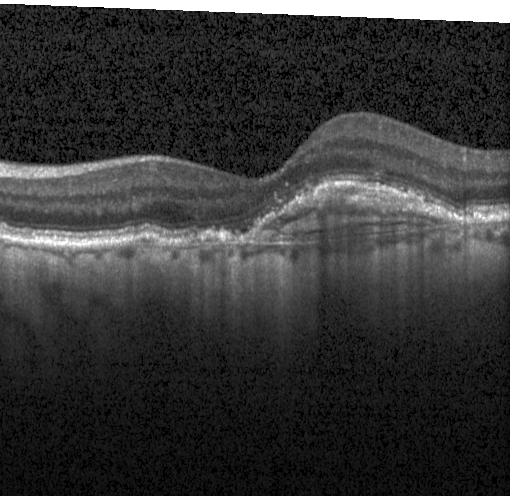 Diagnosis: a choroidal neovascular membrane.